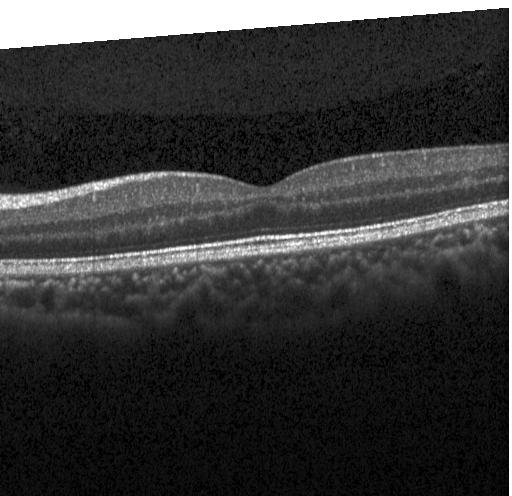
Fovea-centered · OCT line scan · Heidelberg Spectralis. Finding: no CNV, DME, or drusen.